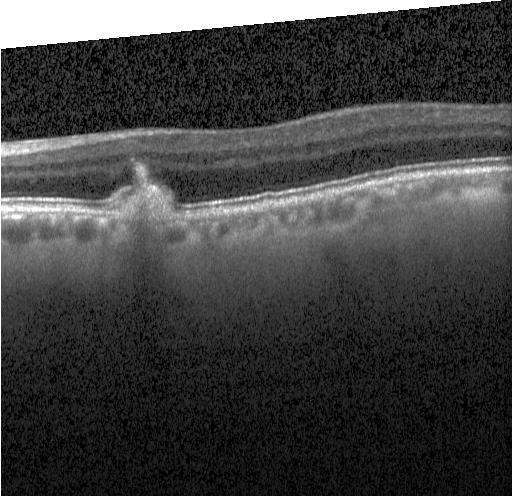

This B-scan demonstrates choroidal neovascularization (CNV).